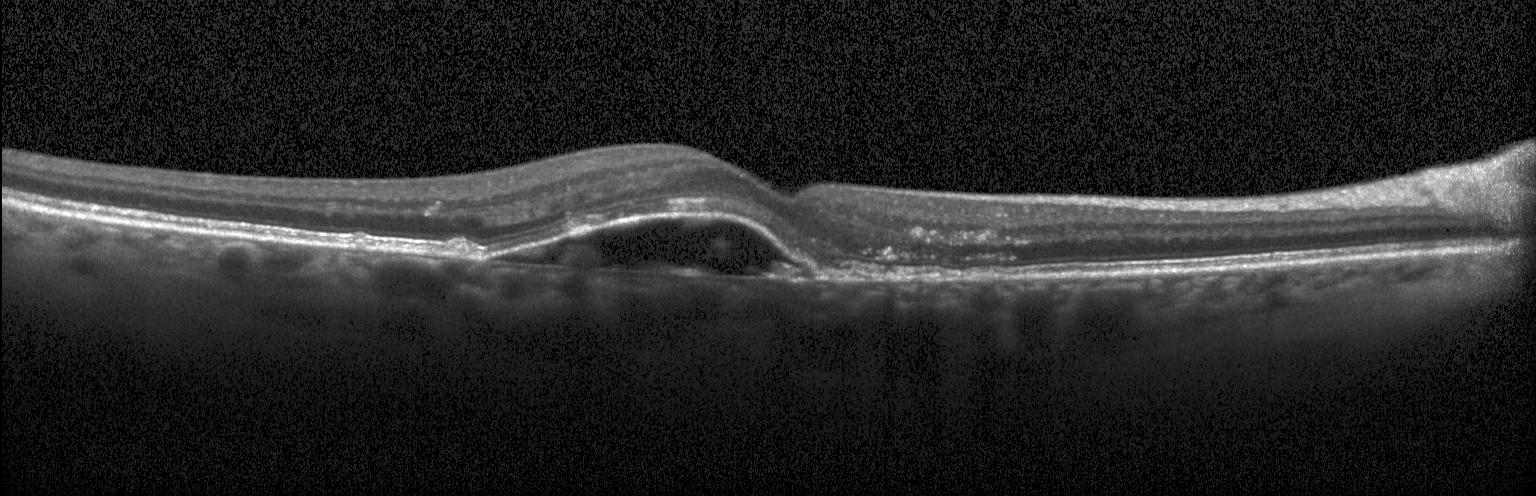 Through the macula; instrument: Heidelberg Spectralis; spectral-domain optical coherence tomography; OCT B-scan.
Assessment: choroidal neovascularization (CNV).